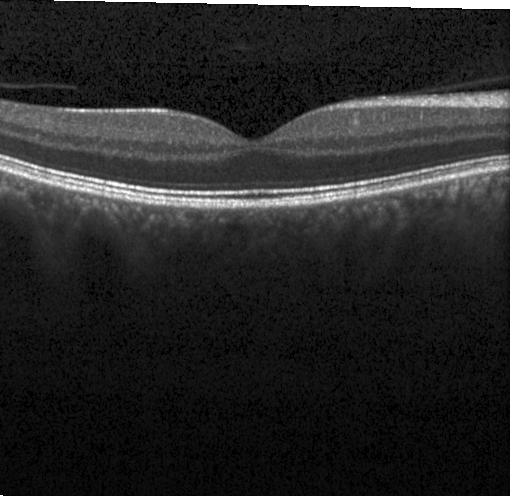
Spectral-domain optical coherence tomography · optical coherence tomography scan · through the macula — Assessment: no evidence of choroidal neovascularization, diabetic macular edema, or drusen.